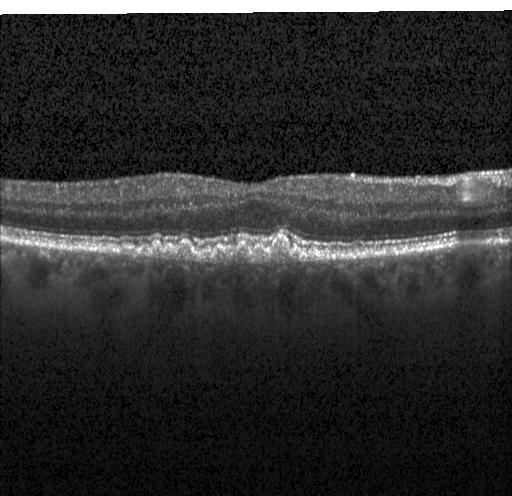

OCT line scan, instrument: Heidelberg Spectralis, spectral-domain OCT, macular scan. The scan shows sub-RPE drusenoid deposits.